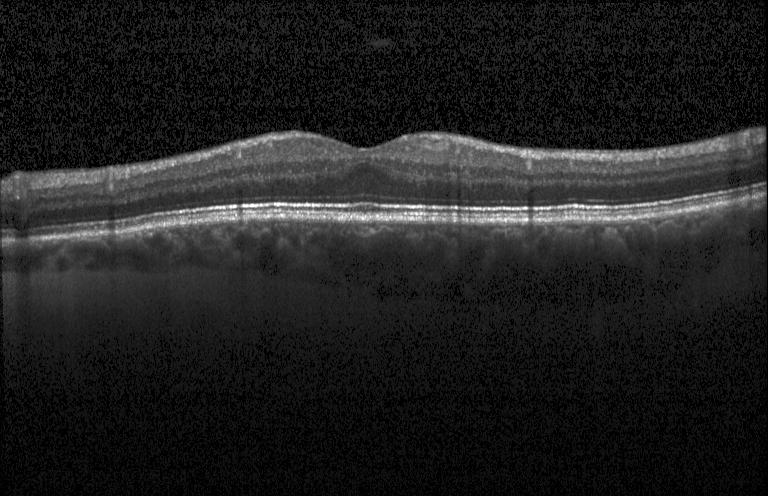 Spectral-domain OCT B-scan: neither choroidal neovascularization, diabetic macular edema, nor drusen.